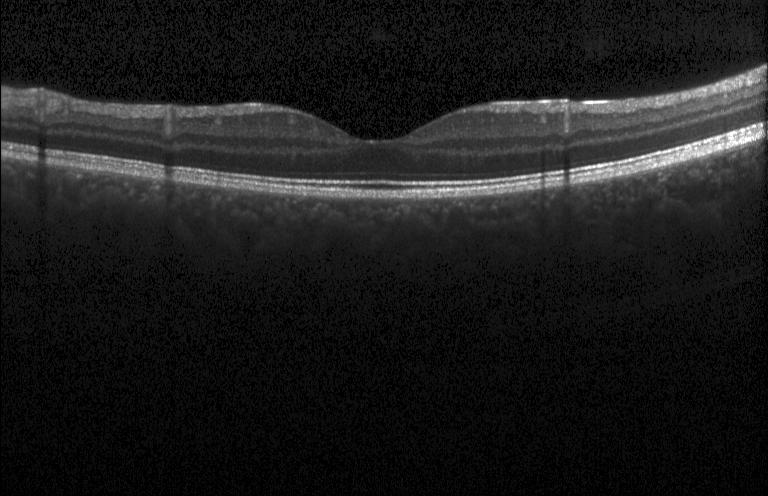

OCT scan showing no CNV, DME, or drusen.